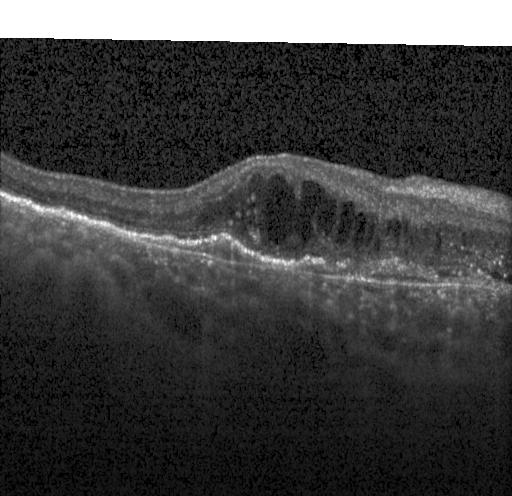

Spectral-domain OCT B-scan: a choroidal neovascular membrane.